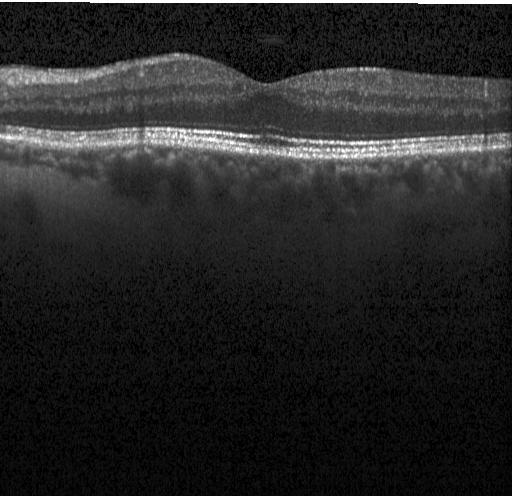
Instrument: Heidelberg Spectralis. Retinal OCT cross-section.
Assessment: no CNV, DME, or drusen.